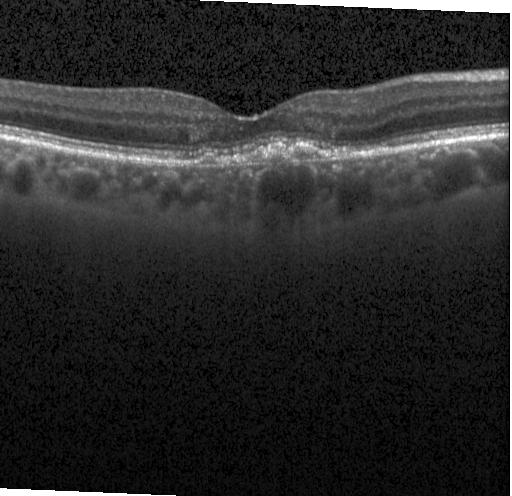
OCT line scan. Spectral-domain OCT. Macular scan — Macular OCT: a choroidal neovascular membrane.